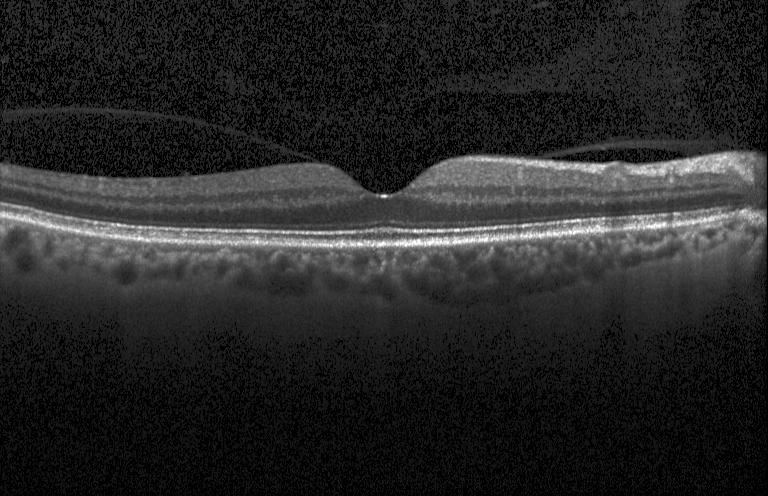
SD-OCT · acquired on a Heidelberg Spectralis · through the macula · optical coherence tomography scan
Dx: no evidence of choroidal neovascularization, diabetic macular edema, or drusen.